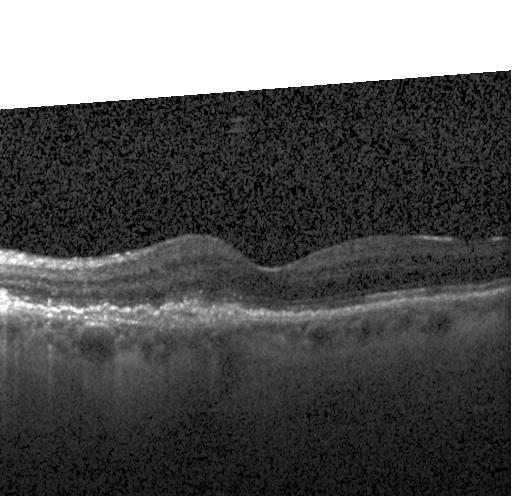 Retinal OCT B-scan. SD-OCT. Diagnosis: a choroidal neovascular membrane.